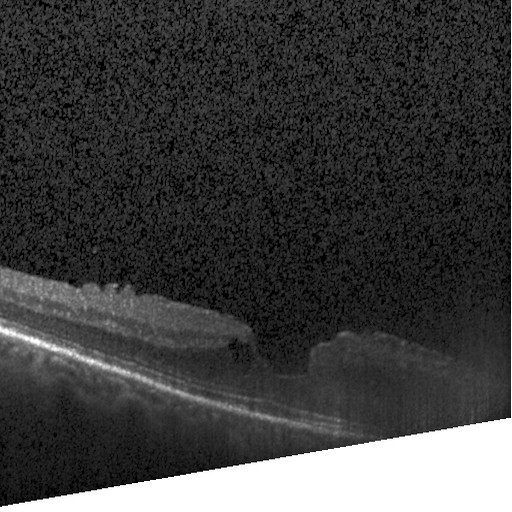
Heidelberg Spectralis OCT system, OCT B-scan, centered on the fovea. The scan shows diabetic macular edema.